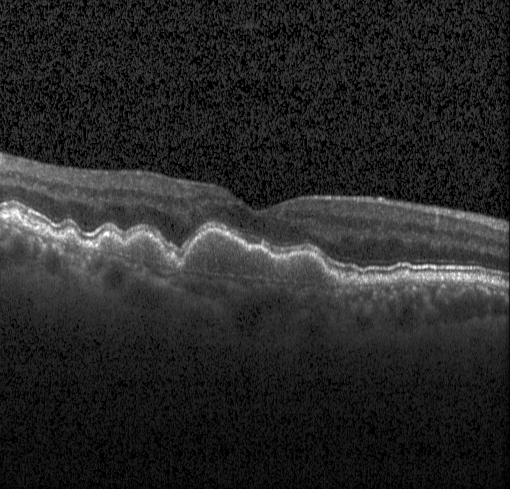

OCT line scan. Diagnosis: multiple drusen.